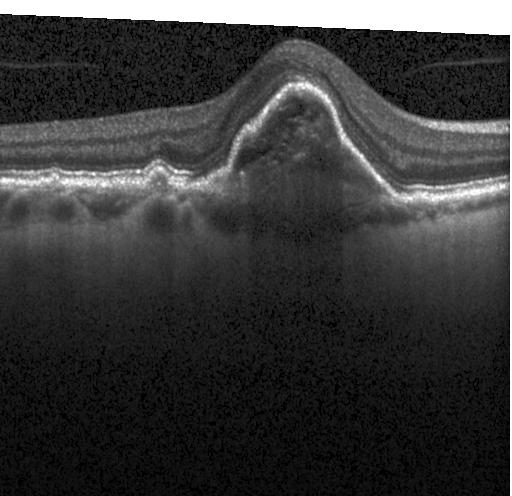

Spectral-domain OCT · macular scan · retinal OCT B-scan — Diagnosis: a choroidal neovascular membrane.